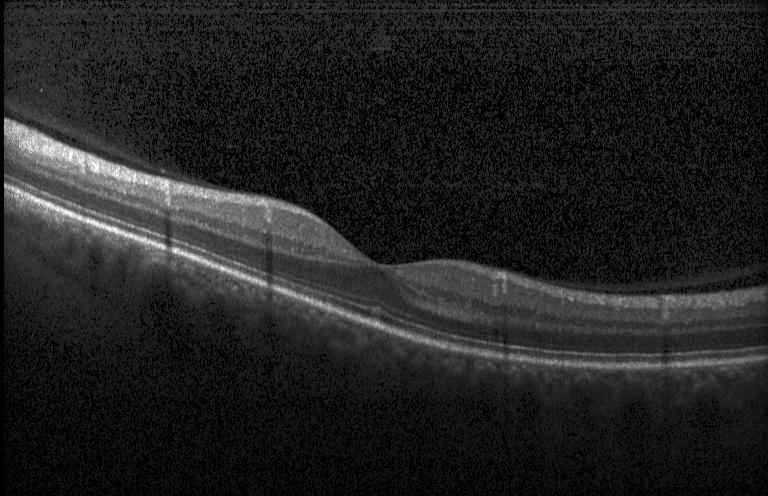

The scan shows neither choroidal neovascularization, diabetic macular edema, nor drusen.